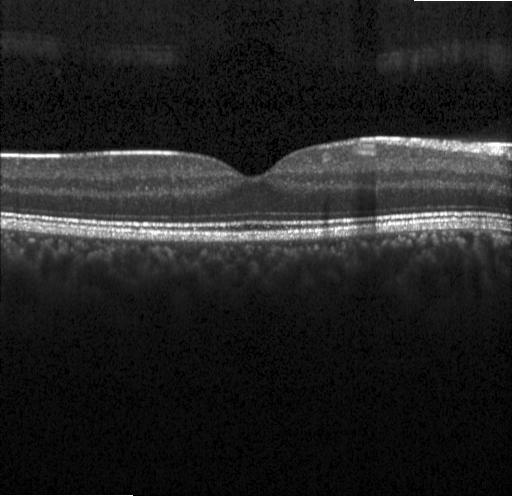

Finding: no choroidal neovascularization, diabetic macular edema, or drusen.